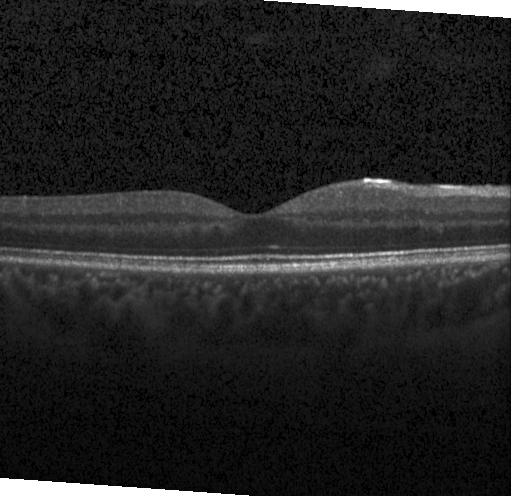
This B-scan demonstrates no choroidal neovascularization, no diabetic macular edema, and no drusen.